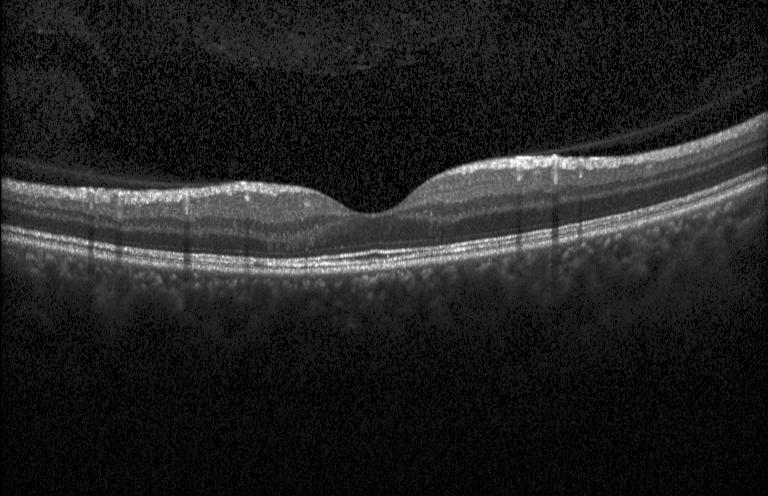 Macular scan, spectral-domain optical coherence tomography, Heidelberg Spectralis OCT system, retinal OCT cross-section.
Macular OCT: neither choroidal neovascularization, diabetic macular edema, nor drusen.